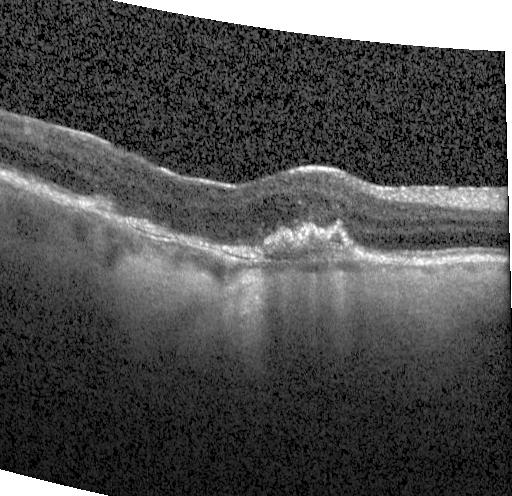 Finding: CNV.